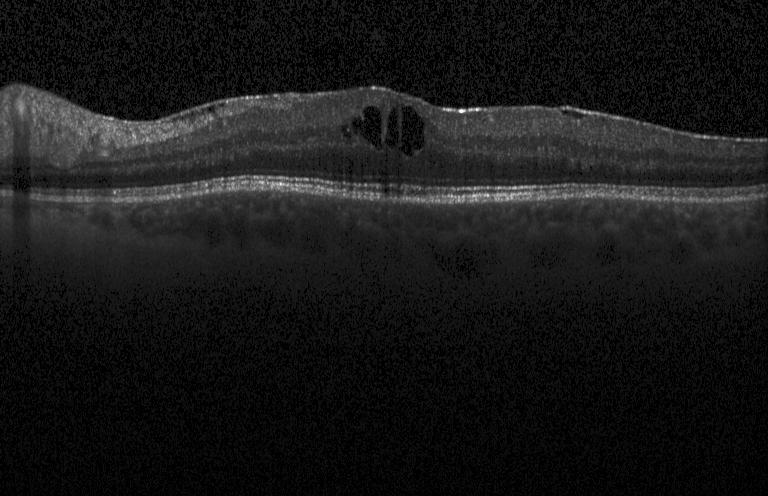

Instrument: Heidelberg Spectralis, OCT line scan. OCT finding: DME.